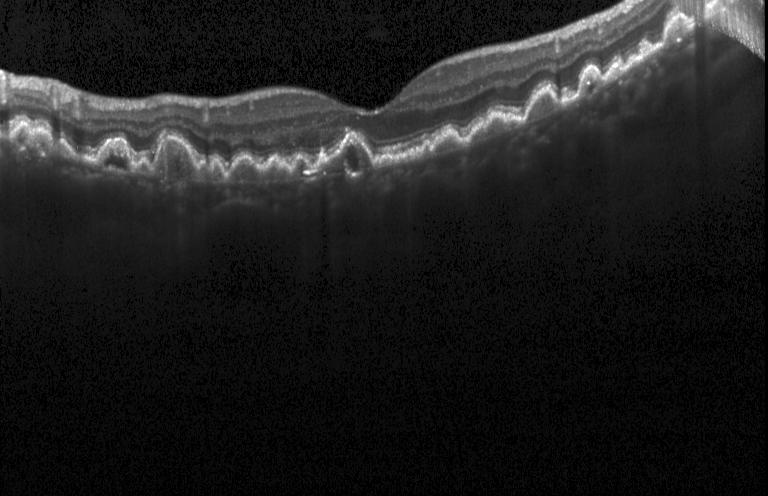
Retinal OCT cross-section; spectral-domain optical coherence tomography; horizontal scan through the fovea. Impression: choroidal neovascularization (CNV).